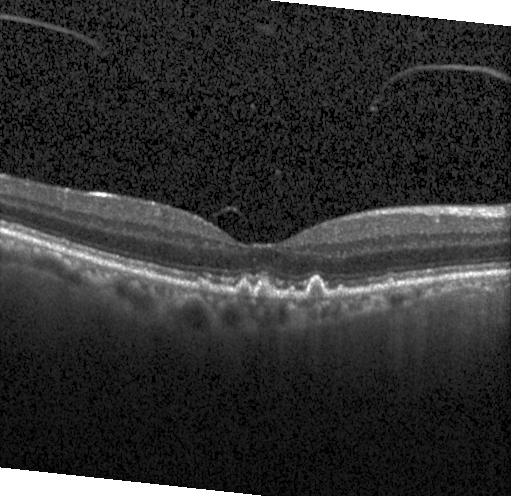

Impression: drusen.